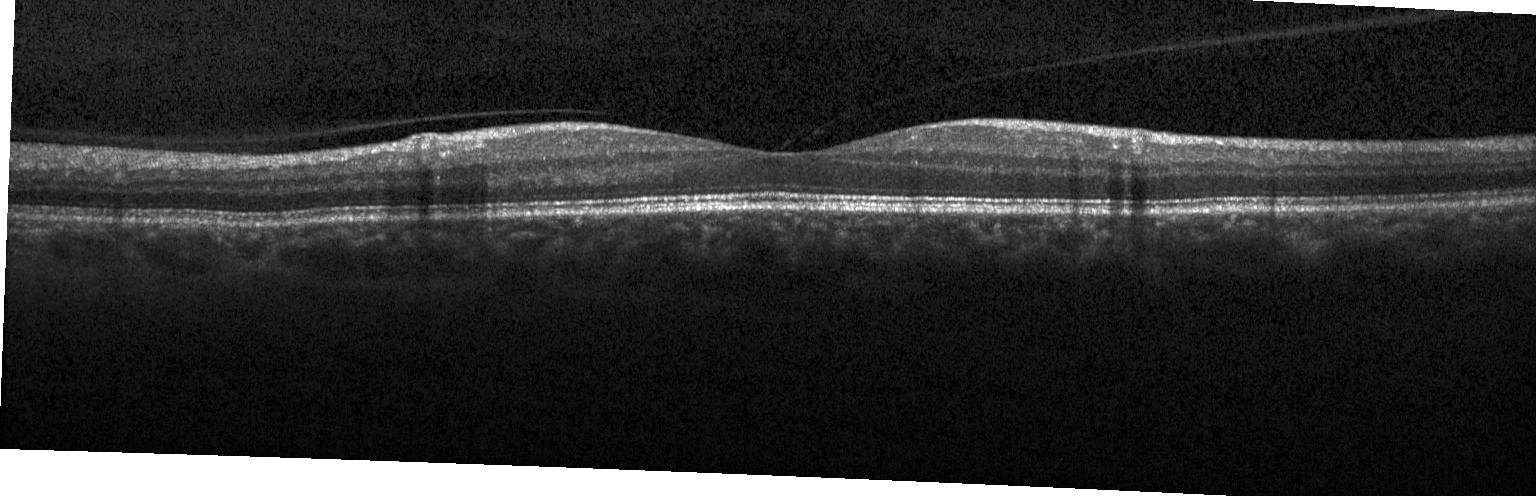 Retinal OCT B-scan. SD-OCT — The scan shows no choroidal neovascularization, diabetic macular edema, or drusen.